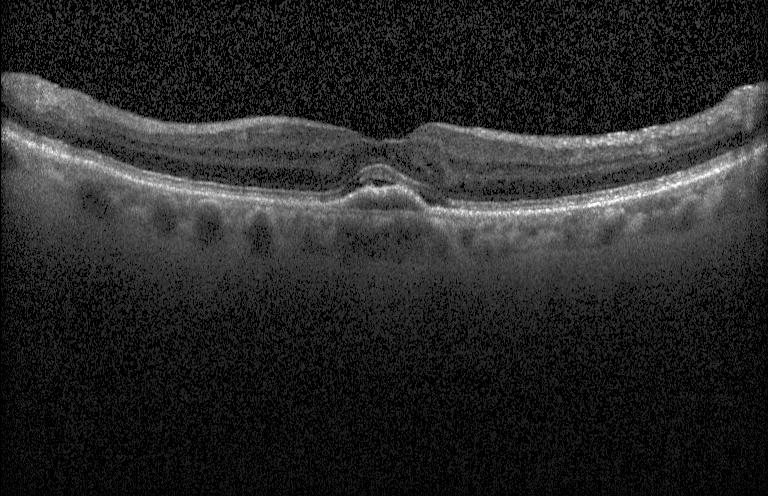
Dx: choroidal neovascularization (CNV).